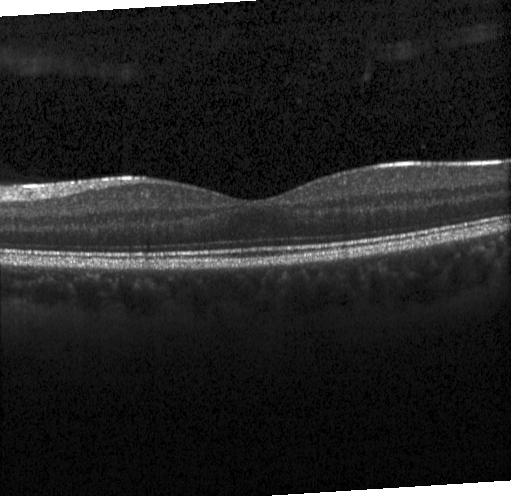 Macular scan; optical coherence tomography scan.
The scan shows neither CNV, DME, nor drusen.